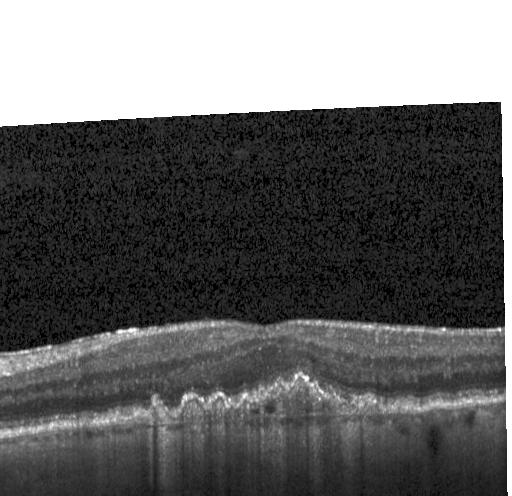 Acquired on a Heidelberg Spectralis · retinal OCT cross-section.
Assessment: a choroidal neovascular membrane.